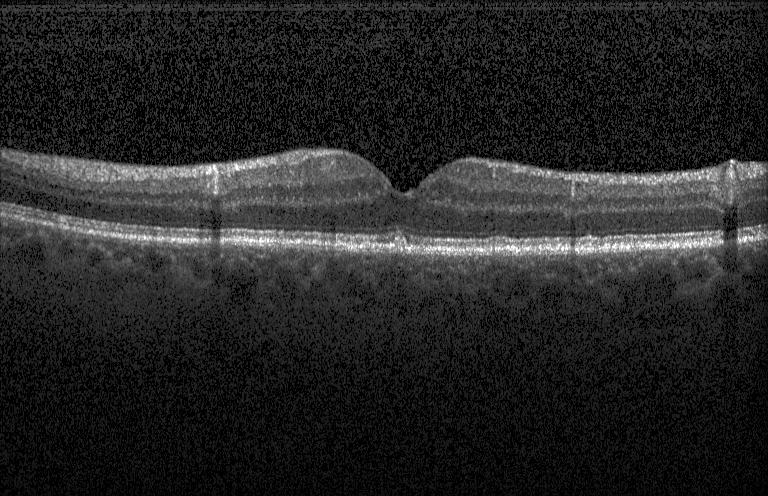

Finding: drusen.